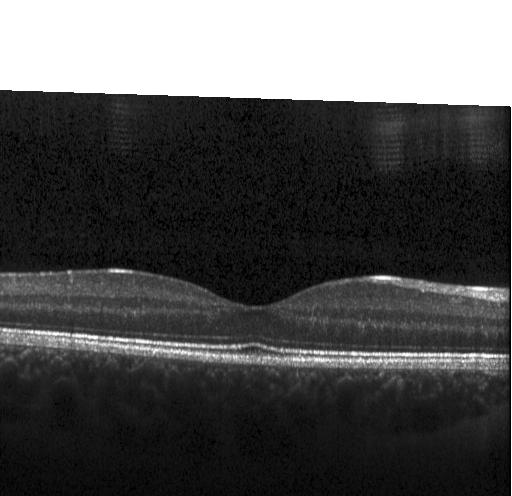

Retinal OCT cross-section showing no CNV, DME, or drusen.